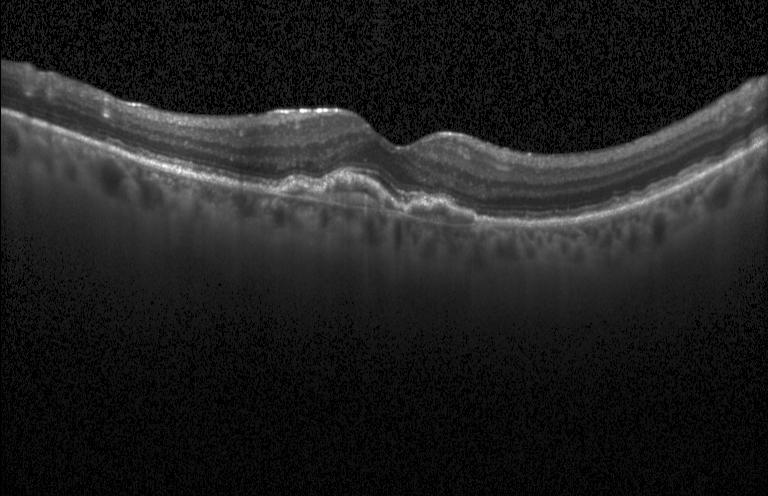
Heidelberg Spectralis, OCT line scan, SD-OCT. The scan shows choroidal neovascularization (CNV).